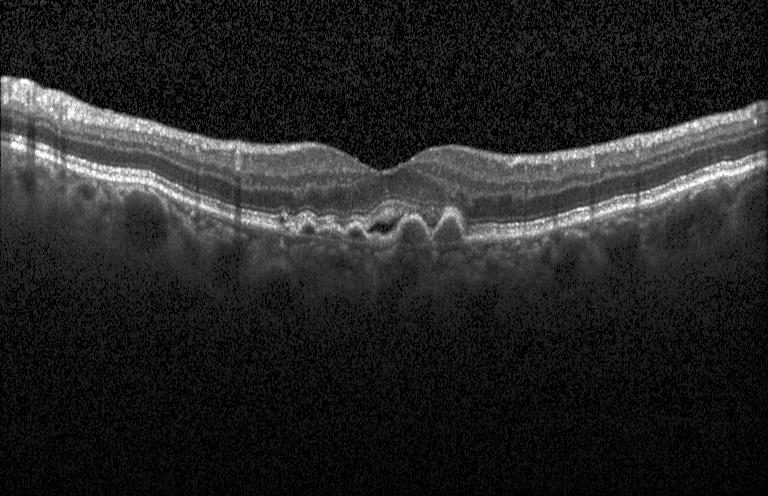
Heidelberg Spectralis OCT system · through the macula · optical coherence tomography B-scan — This B-scan demonstrates choroidal neovascularization.